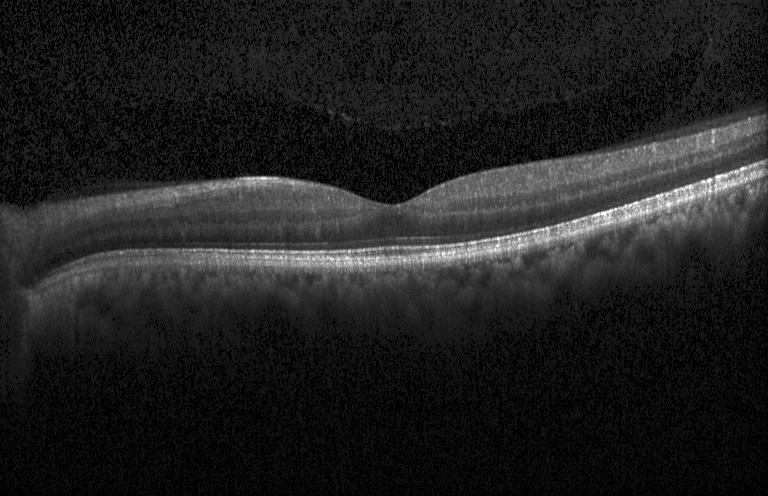
Macular OCT demonstrating no choroidal neovascularization, no diabetic macular edema, and no drusen.